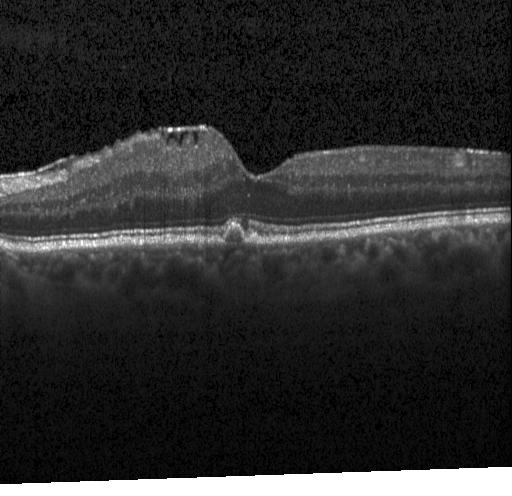
Optical coherence tomography B-scan. Macular OCT: drusen.